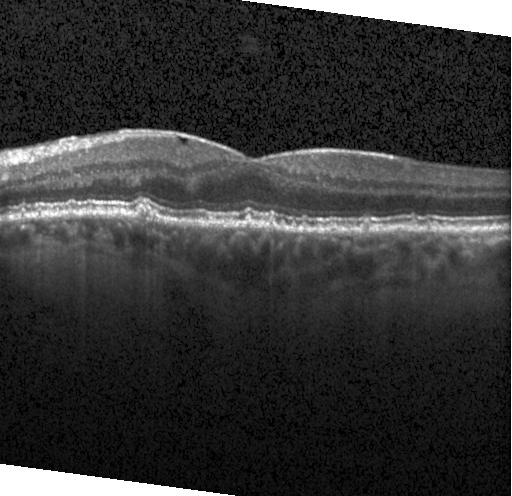 Horizontal scan through the fovea. Spectral-domain optical coherence tomography. OCT B-scan.
Finding: sub-RPE drusenoid deposits.